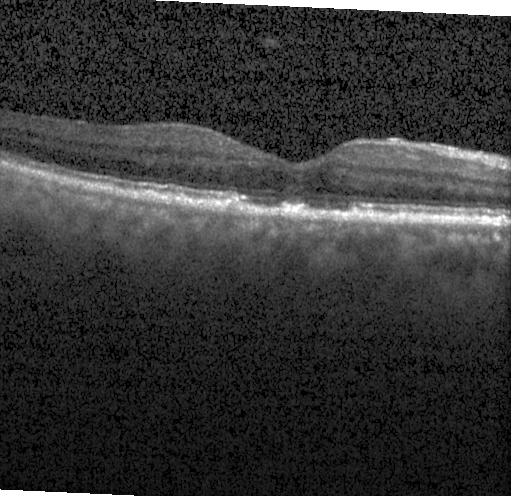
OCT line scan. Diagnosis: multiple drusen.